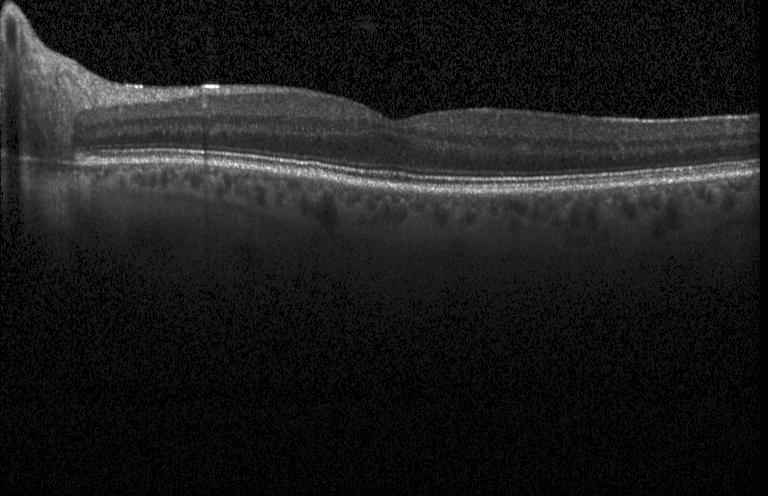

Fovea-centered; spectral-domain OCT; OCT B-scan.
Impression: no evidence of choroidal neovascularization, diabetic macular edema, or drusen.